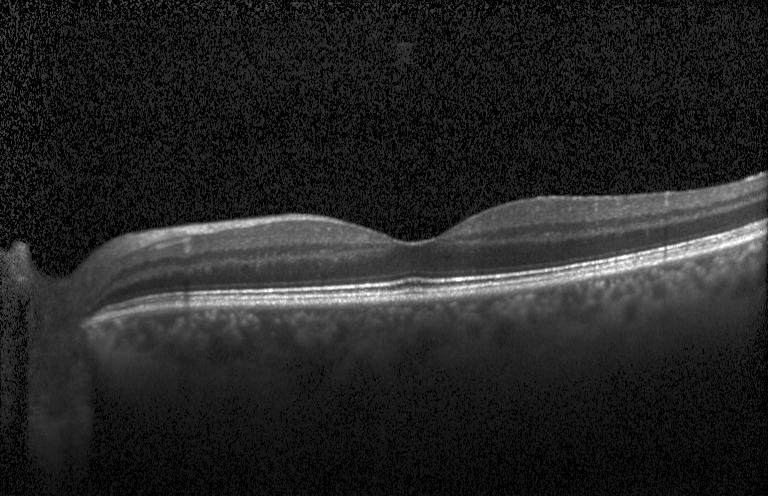 Assessment: no choroidal neovascularization, no diabetic macular edema, and no drusen.